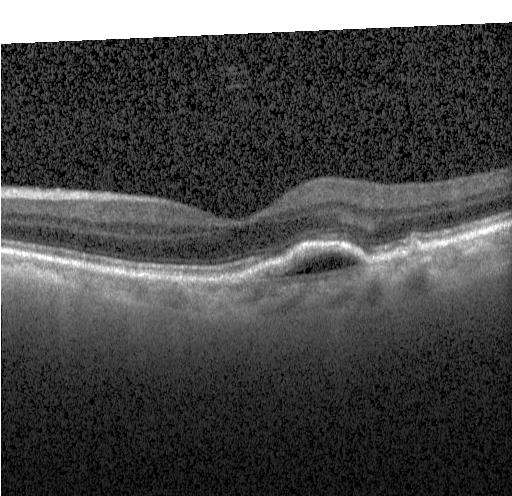

Retinal OCT B-scan, centered on the fovea — Diagnosis: CNV.